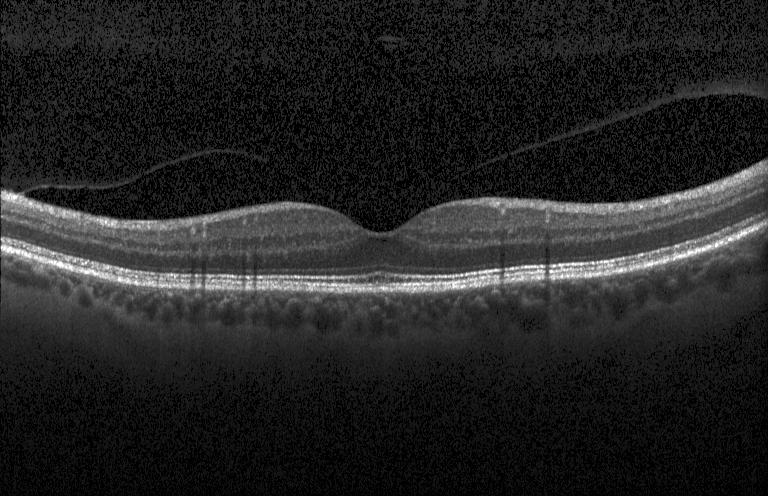
Finding: no choroidal neovascularization, diabetic macular edema, or drusen.